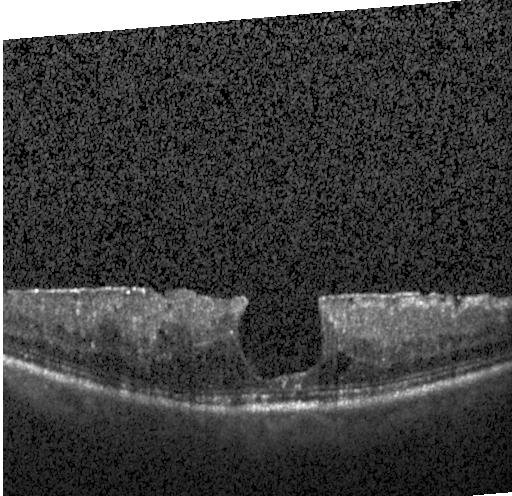

Optical coherence tomography B-scan — Impression: DME.